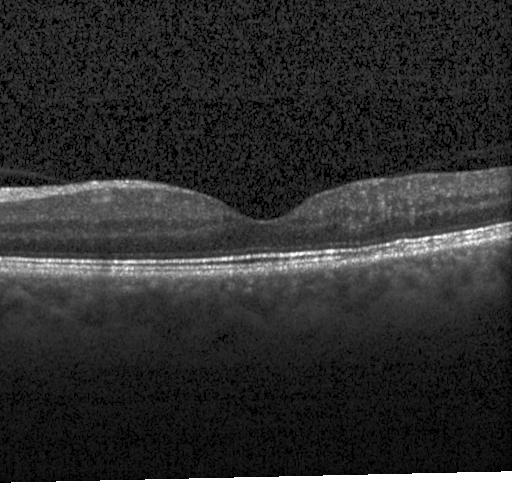

Spectral-domain OCT; retinal OCT cross-section; fovea-centered; instrument: Heidelberg Spectralis
Finding: neither choroidal neovascularization, diabetic macular edema, nor drusen.